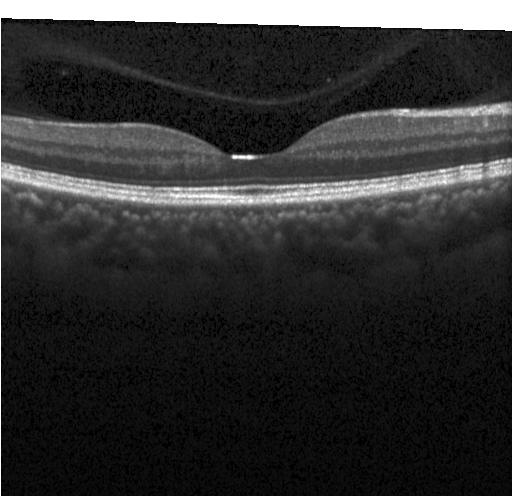 OCT B-scan. Macular OCT: no CNV, DME, or drusen.